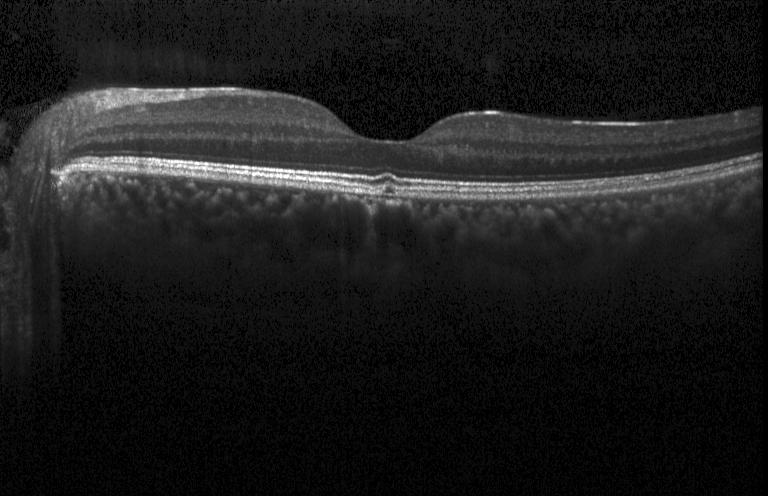 The scan shows neither CNV, DME, nor drusen.